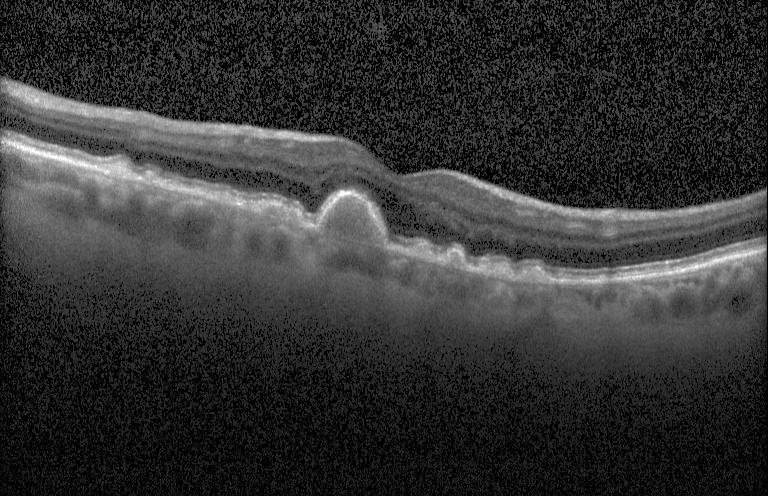

Optical coherence tomography scan.
Diagnosis: drusen.